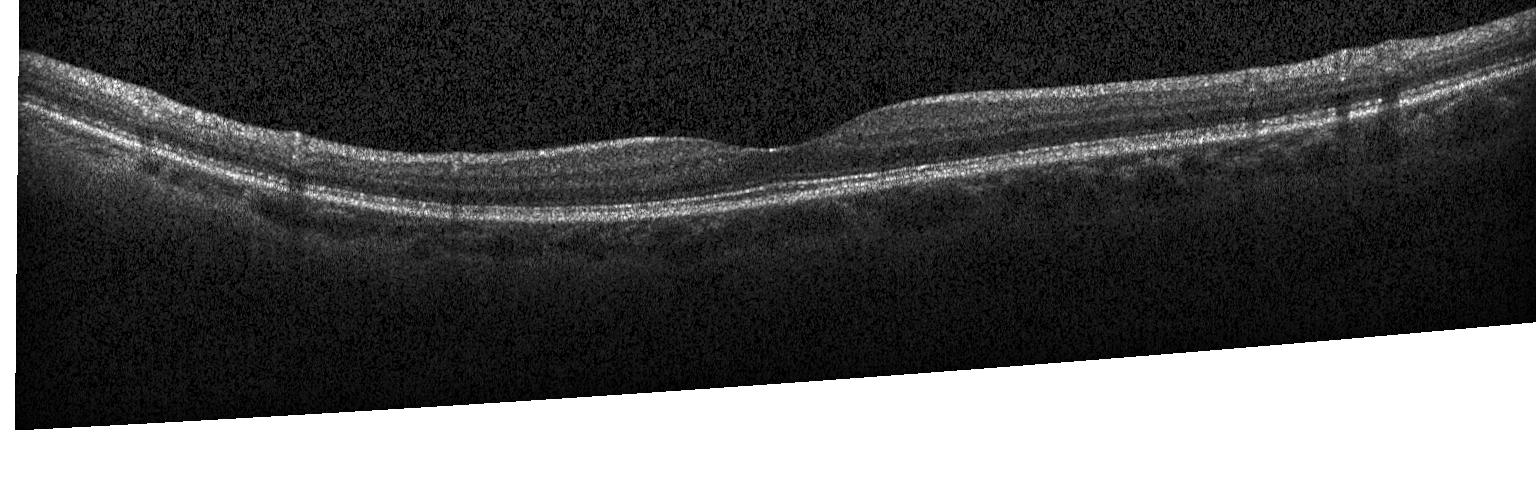

Macular scan, optical coherence tomography scan, spectral-domain OCT.
OCT finding: no choroidal neovascularization, diabetic macular edema, or drusen.